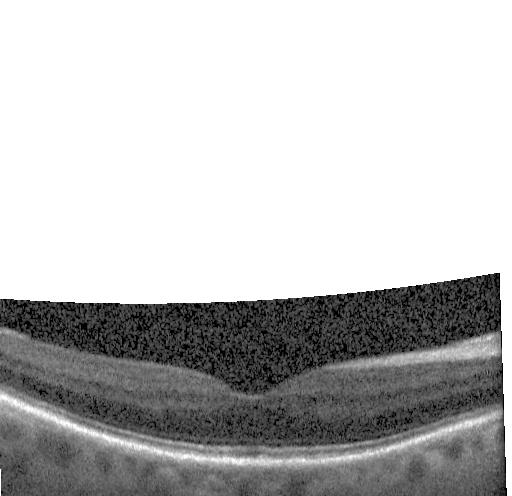 Spectral-domain optical coherence tomography; retinal OCT B-scan. Finding: neither CNV, DME, nor drusen.